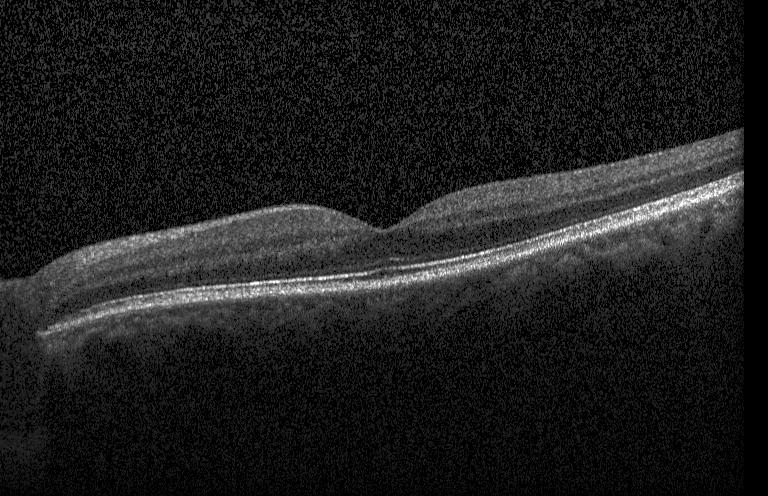 Finding: no choroidal neovascularization, no diabetic macular edema, and no drusen.